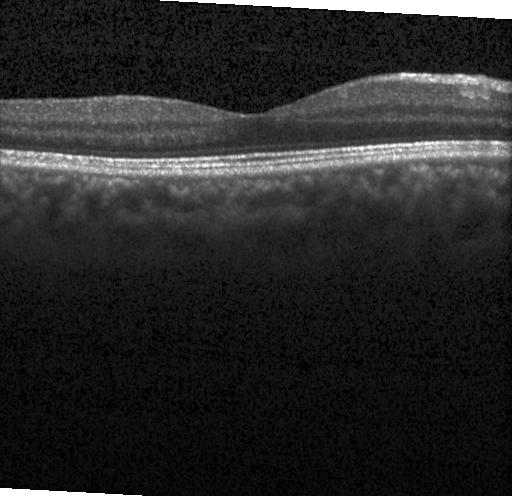
Diagnosis: no choroidal neovascularization, diabetic macular edema, or drusen.